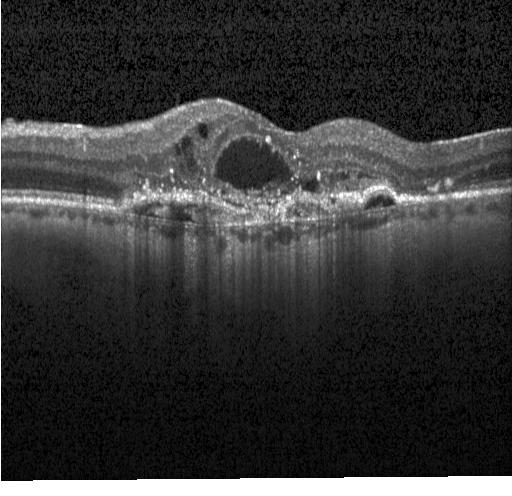
Acquired on a Heidelberg Spectralis · OCT line scan.
Diagnosis: choroidal neovascularization (CNV).